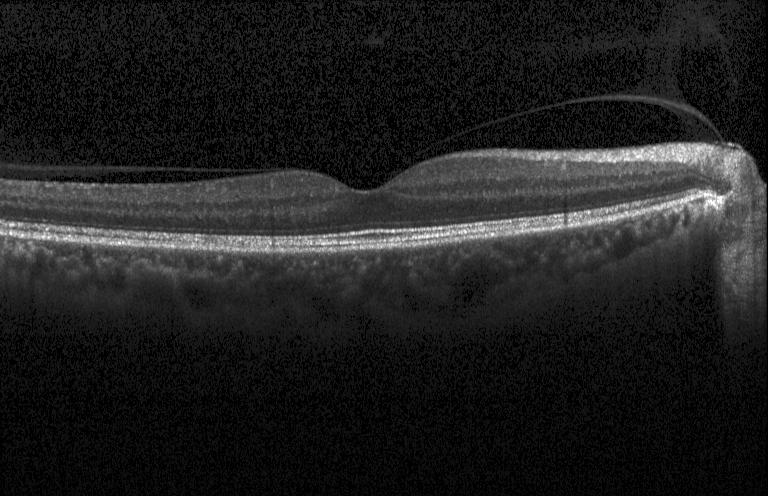
SD-OCT. Retinal OCT B-scan. Heidelberg Spectralis OCT system — Macular OCT: no evidence of choroidal neovascularization, diabetic macular edema, or drusen.